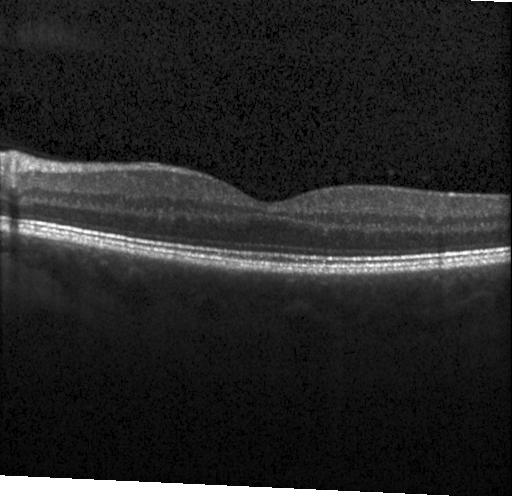
Heidelberg Spectralis OCT system · retinal OCT cross-section · horizontal scan through the fovea · spectral-domain optical coherence tomography.
Finding: neither choroidal neovascularization, diabetic macular edema, nor drusen.